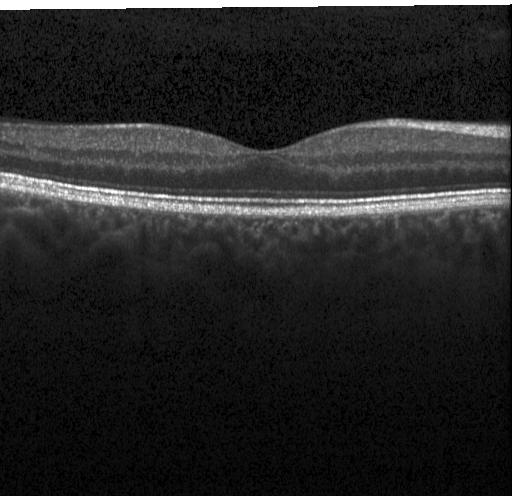

OCT B-scan.
Diagnosis: no CNV, DME, or drusen.